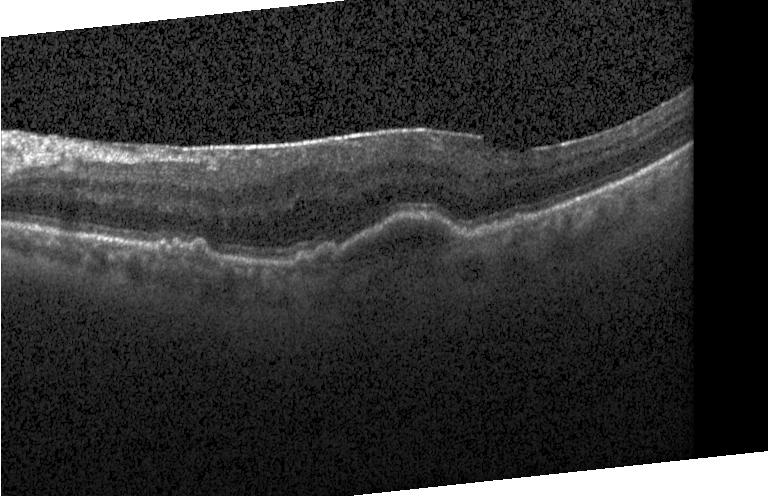
Optical coherence tomography B-scan; acquired on a Heidelberg Spectralis; SD-OCT.
The scan shows choroidal neovascularization.